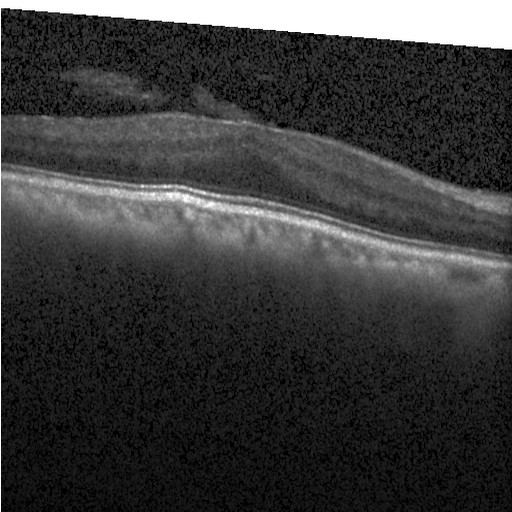 Through the macula; OCT B-scan; SD-OCT
This B-scan demonstrates diabetic macular edema (DME).